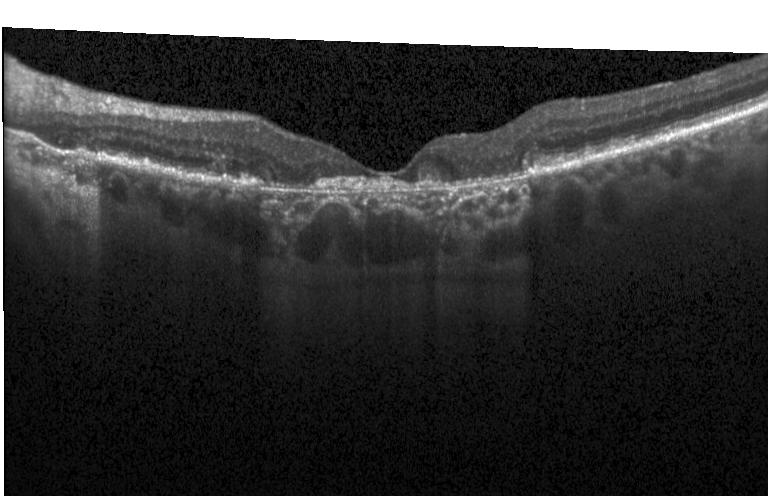 Centered on the fovea. Acquired on a Heidelberg Spectralis. Spectral-domain OCT. Retinal OCT B-scan. Macular OCT: CNV.